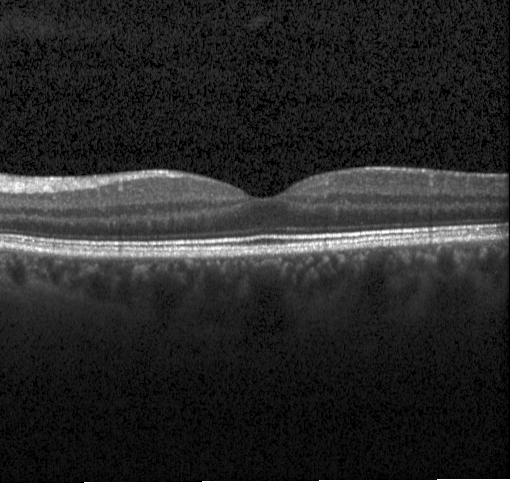
Horizontal scan through the fovea. Retinal OCT cross-section.
No evidence of CNV, DME, or drusen.